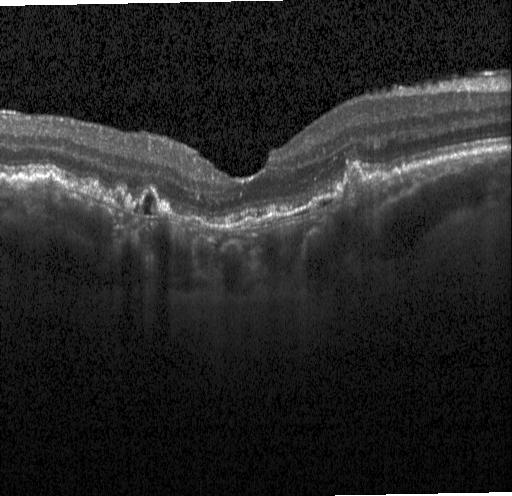
This B-scan demonstrates choroidal neovascularization (CNV).